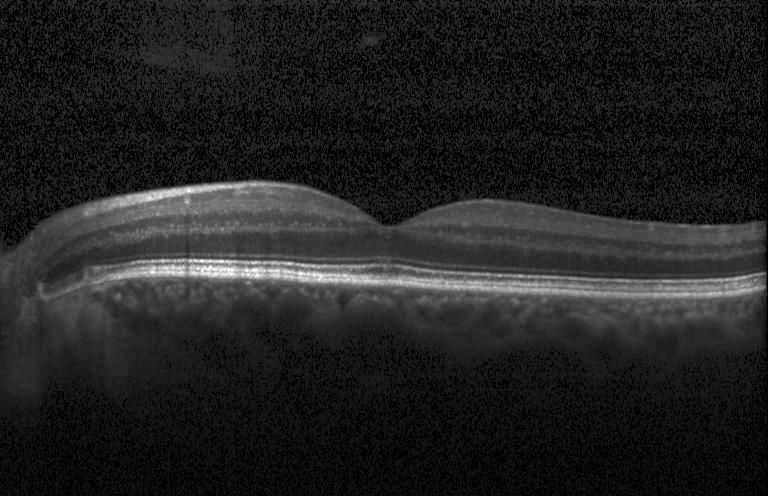
The scan shows no choroidal neovascularization, diabetic macular edema, or drusen.